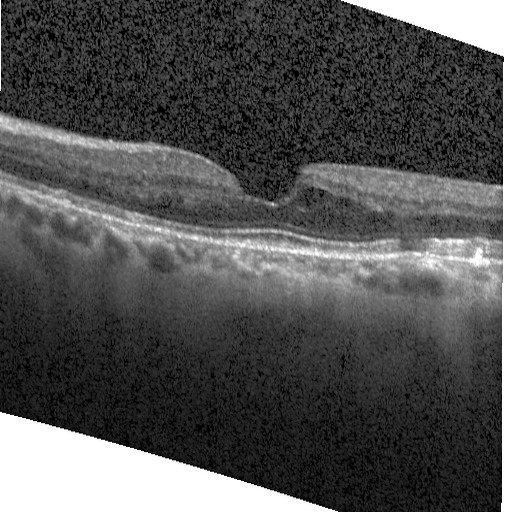
Acquired on a Heidelberg Spectralis; through the macula; spectral-domain OCT; OCT B-scan — Diagnosis: diabetic macular edema.